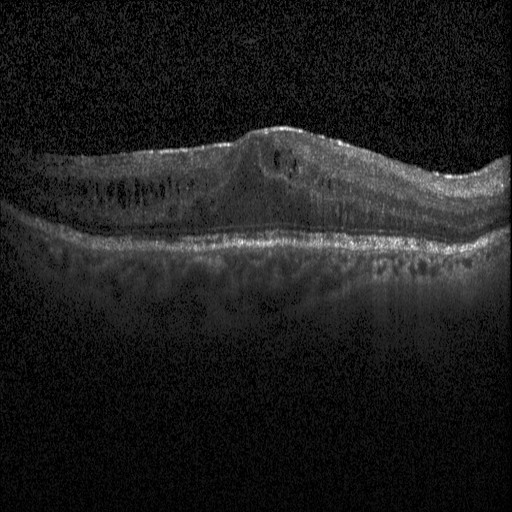
Dx: diabetic macular edema.